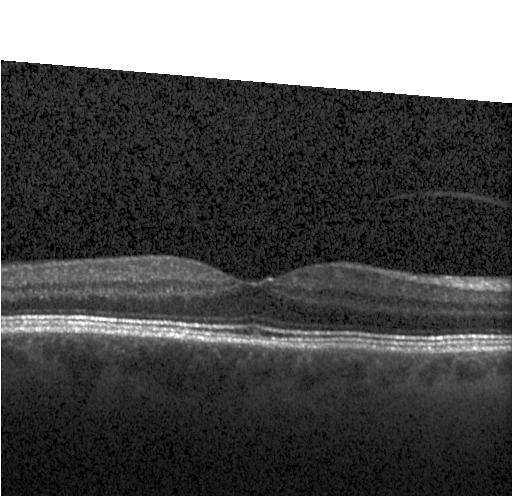

Heidelberg Spectralis, OCT B-scan
Diagnosis: neither choroidal neovascularization, diabetic macular edema, nor drusen.